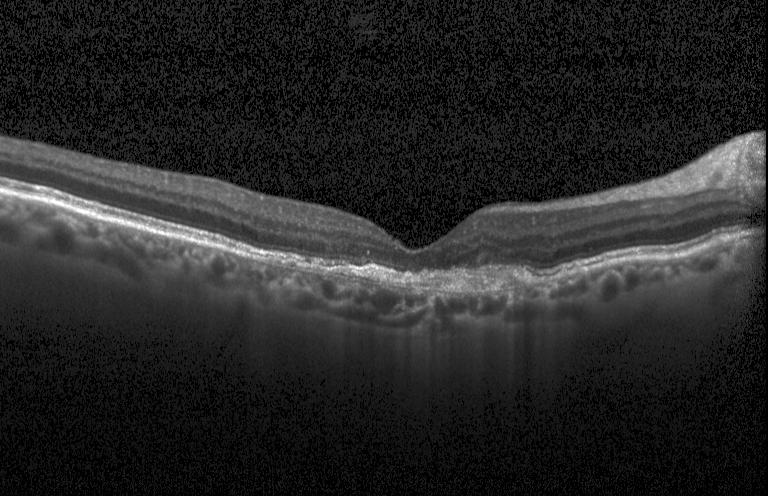
Spectral-domain optical coherence tomography. Optical coherence tomography B-scan. Fovea-centered.
Finding: a choroidal neovascular membrane.